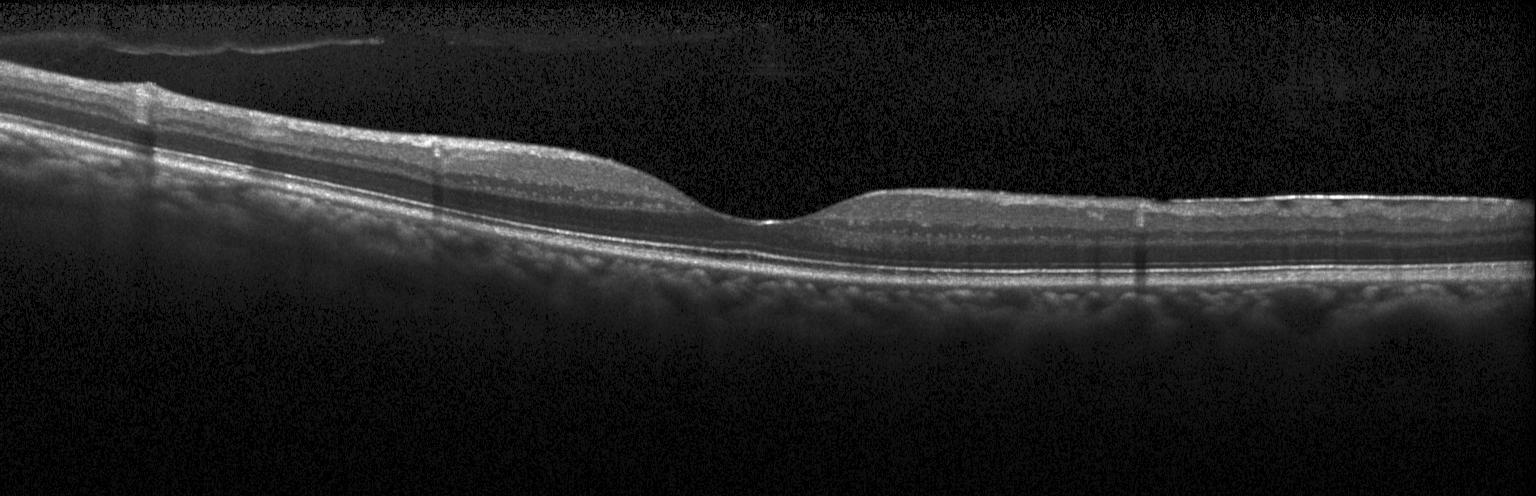
Diagnosis: neither choroidal neovascularization, diabetic macular edema, nor drusen.